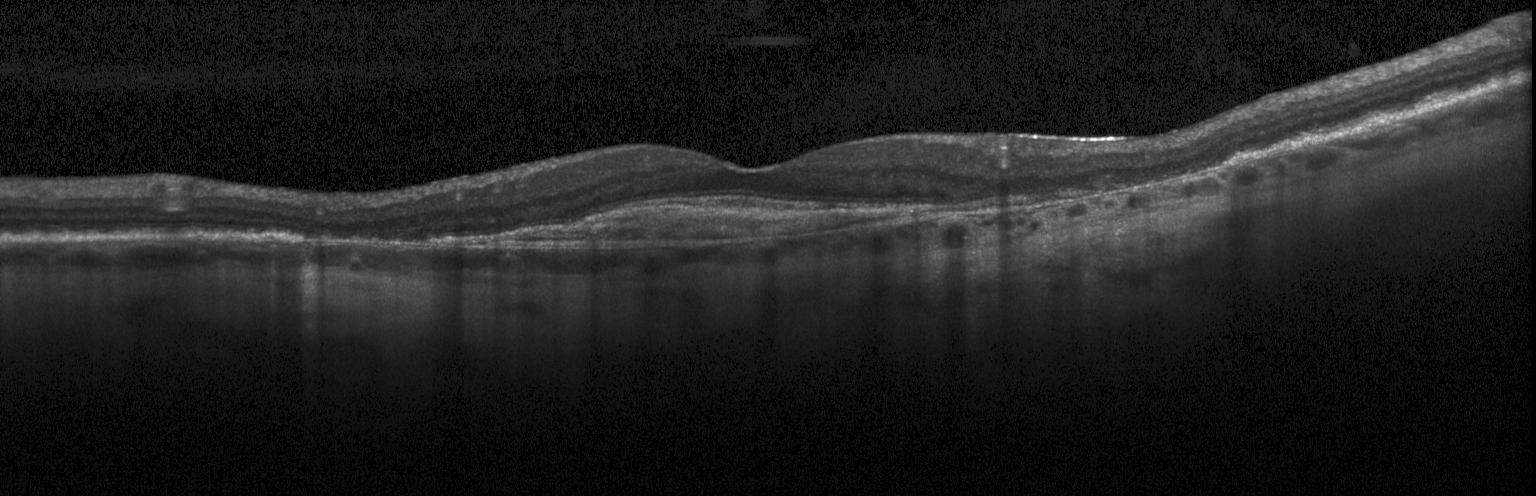
Diagnosis: a choroidal neovascular membrane.